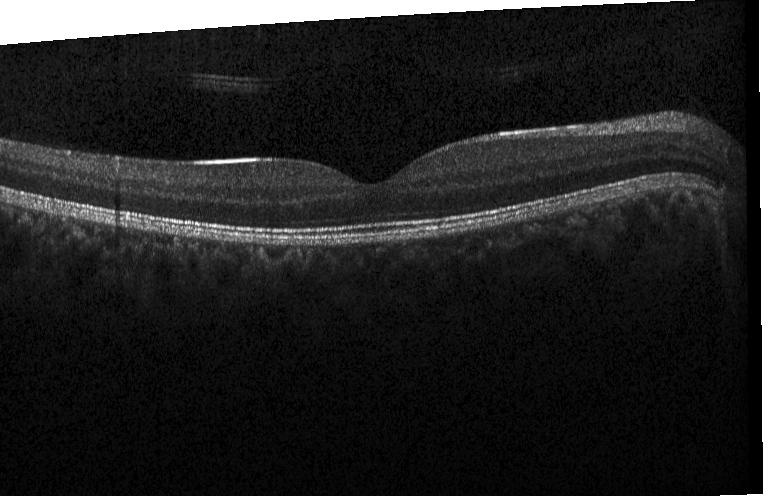 Retinal OCT B-scan — Impression: no choroidal neovascularization, diabetic macular edema, or drusen.